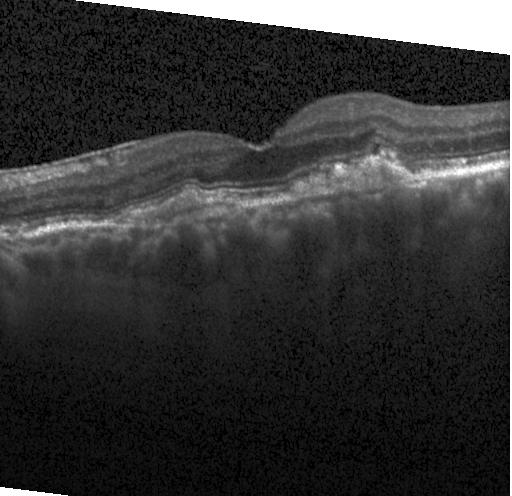 Horizontal scan through the fovea. SD-OCT. Acquired on a Heidelberg Spectralis. Retinal OCT B-scan
Impression: choroidal neovascularization (CNV).